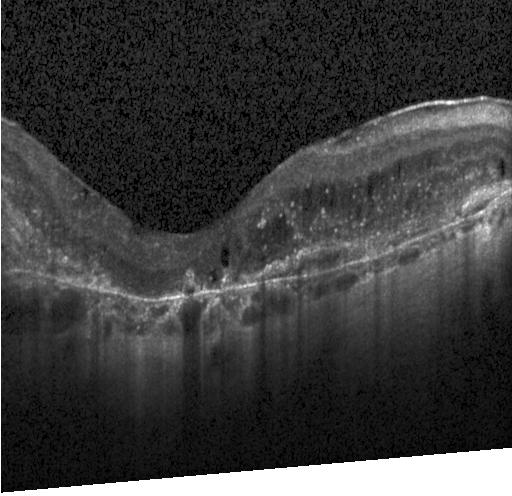
Retinal OCT B-scan; Heidelberg Spectralis
Impression: a choroidal neovascular membrane.